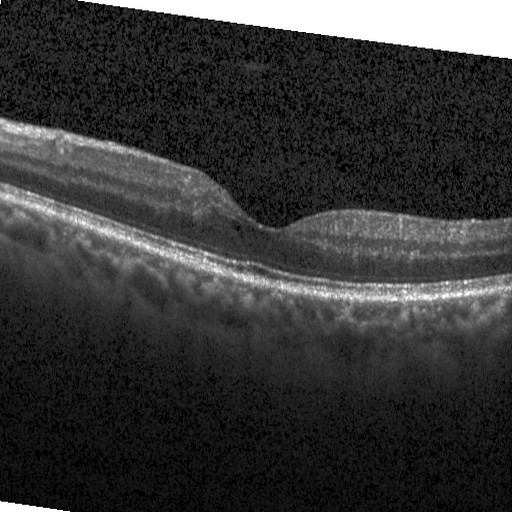 Diagnosis: diabetic macular edema (DME).